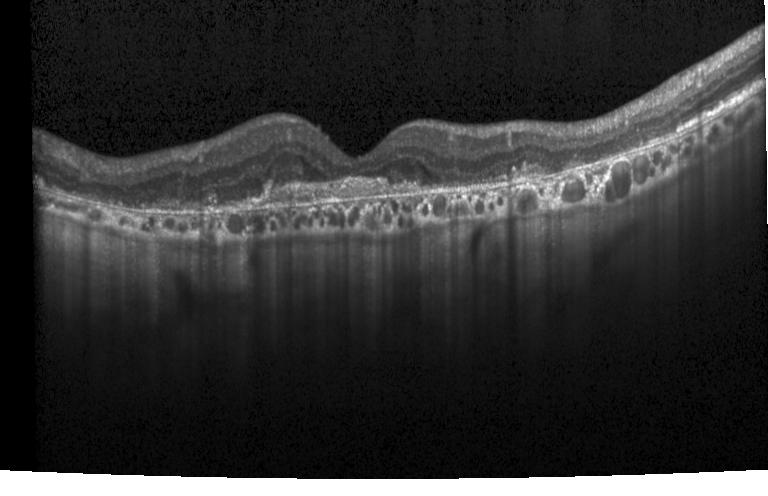 Retinal OCT cross-section showing a choroidal neovascular membrane.